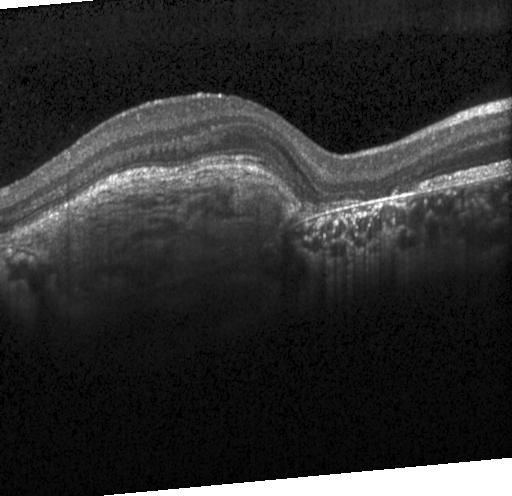

Spectral-domain OCT B-scan: a choroidal neovascular membrane.